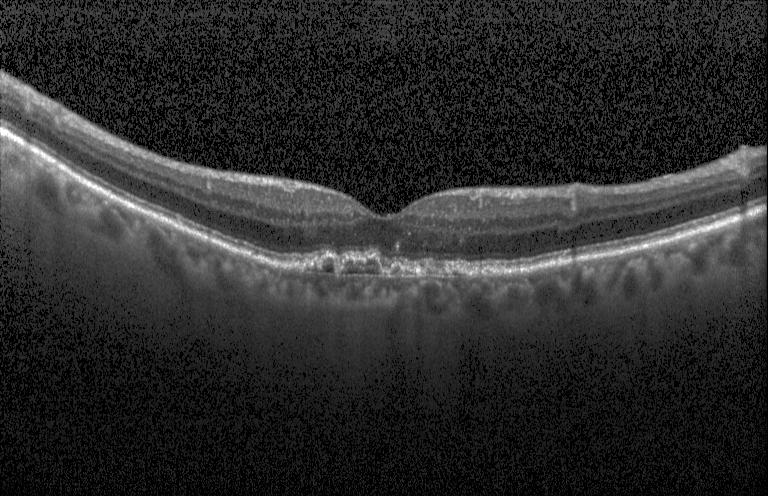 SD-OCT · OCT B-scan
Dx: choroidal neovascularization.